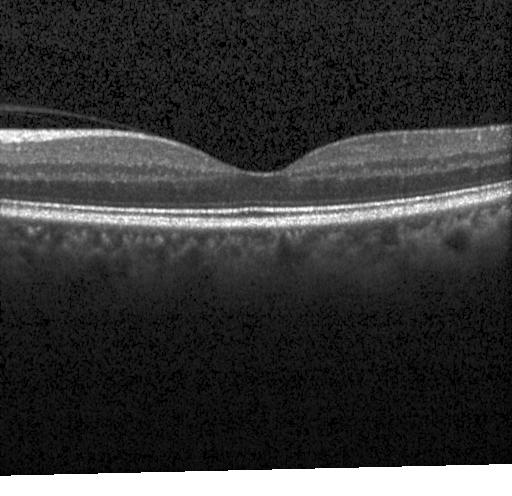

Optical coherence tomography scan, spectral-domain OCT, instrument: Heidelberg Spectralis
Diagnosis: no choroidal neovascularization, no diabetic macular edema, and no drusen.